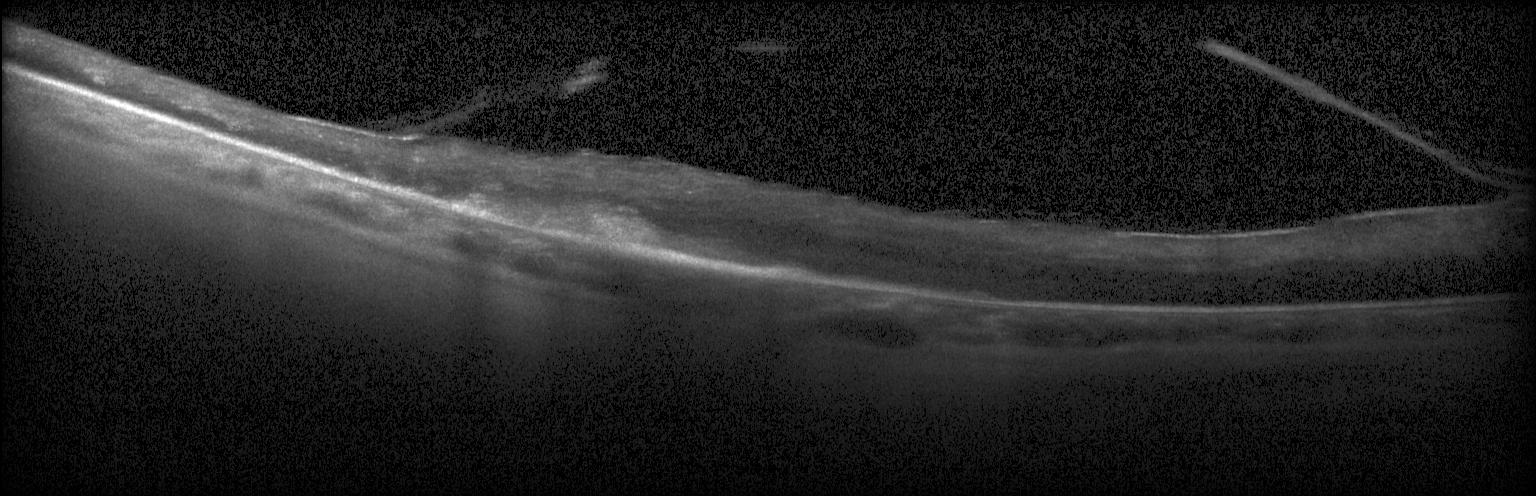
Optical coherence tomography scan · fovea-centered
Assessment: choroidal neovascularization (CNV).